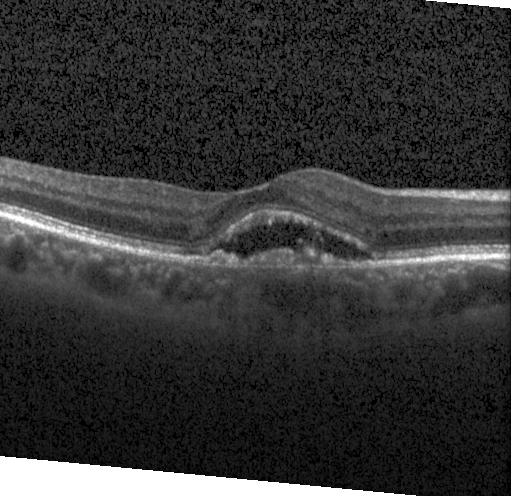
Acquired on a Heidelberg Spectralis, fovea-centered, spectral-domain optical coherence tomography, OCT B-scan. Dx: choroidal neovascularization.